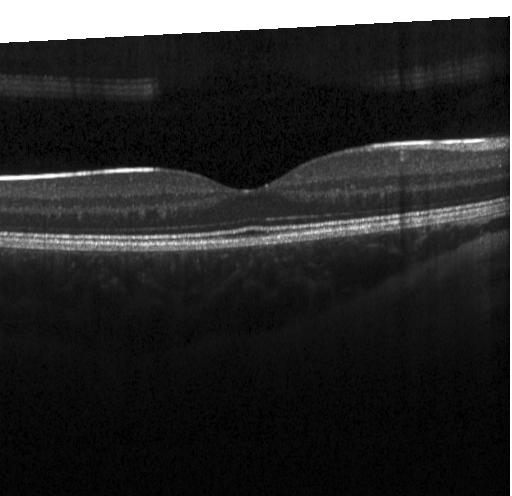 This B-scan demonstrates no evidence of CNV, DME, or drusen.